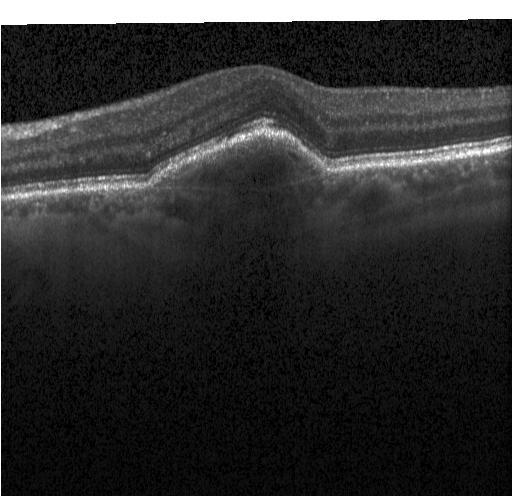 Spectral-domain OCT B-scan: CNV.